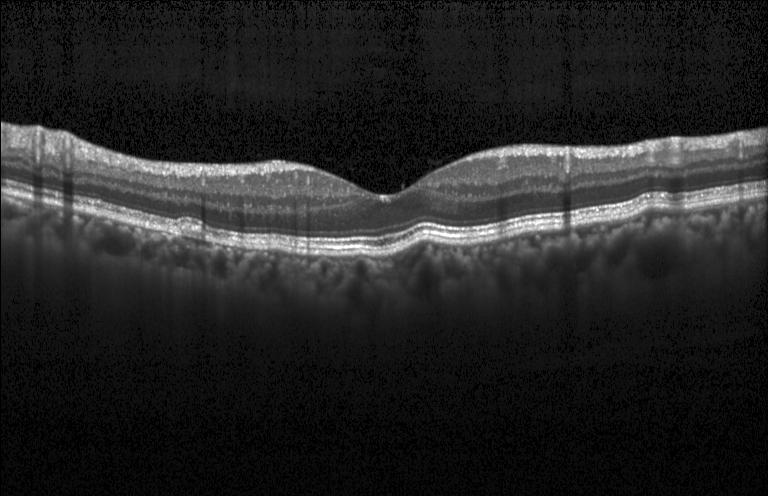 Multiple drusen.